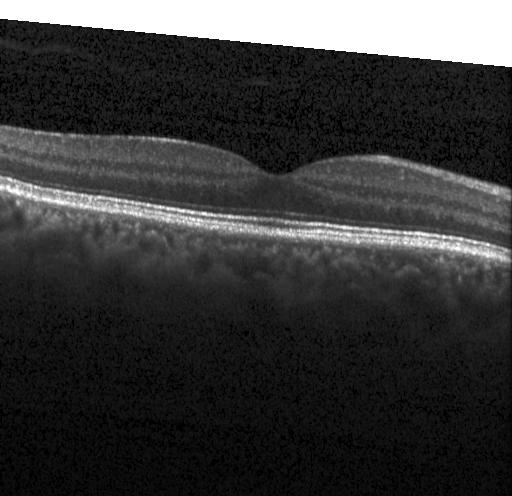
This B-scan demonstrates no choroidal neovascularization, no diabetic macular edema, and no drusen.